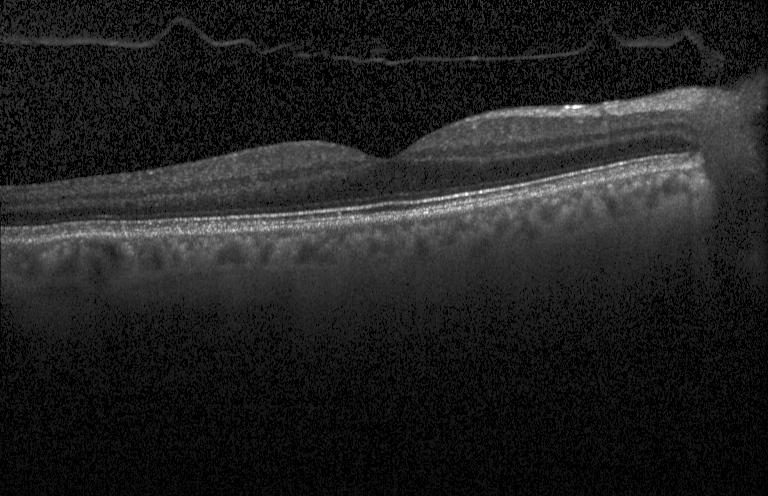
Through the macula; retinal OCT B-scan
Assessment: no choroidal neovascularization, no diabetic macular edema, and no drusen.